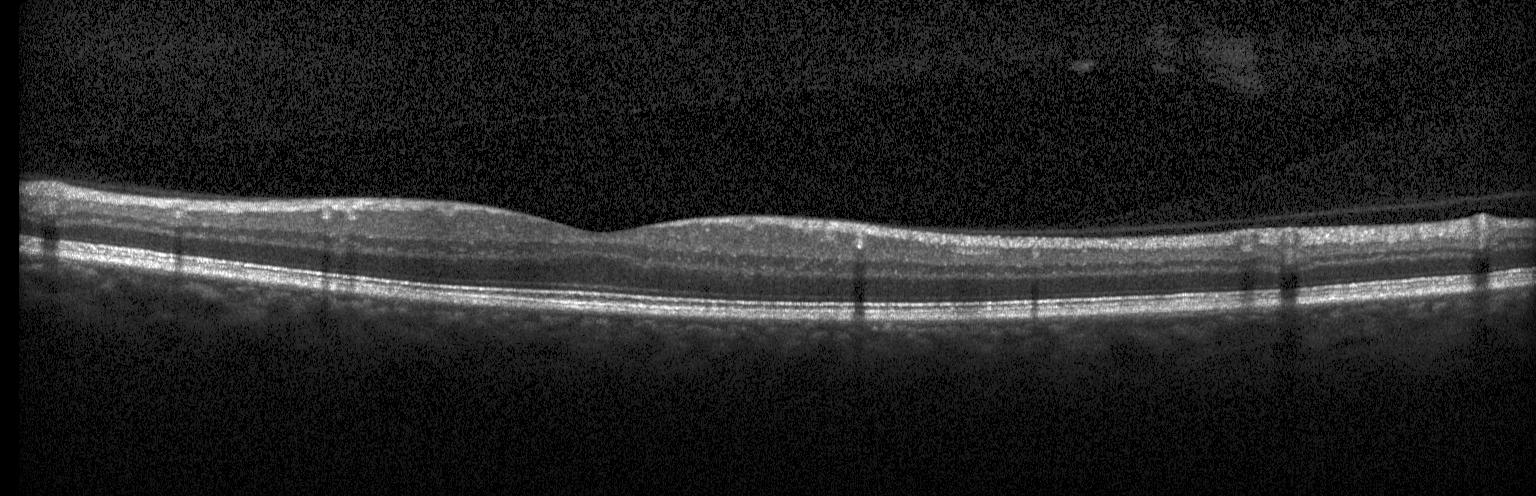

No evidence of choroidal neovascularization, diabetic macular edema, or drusen.